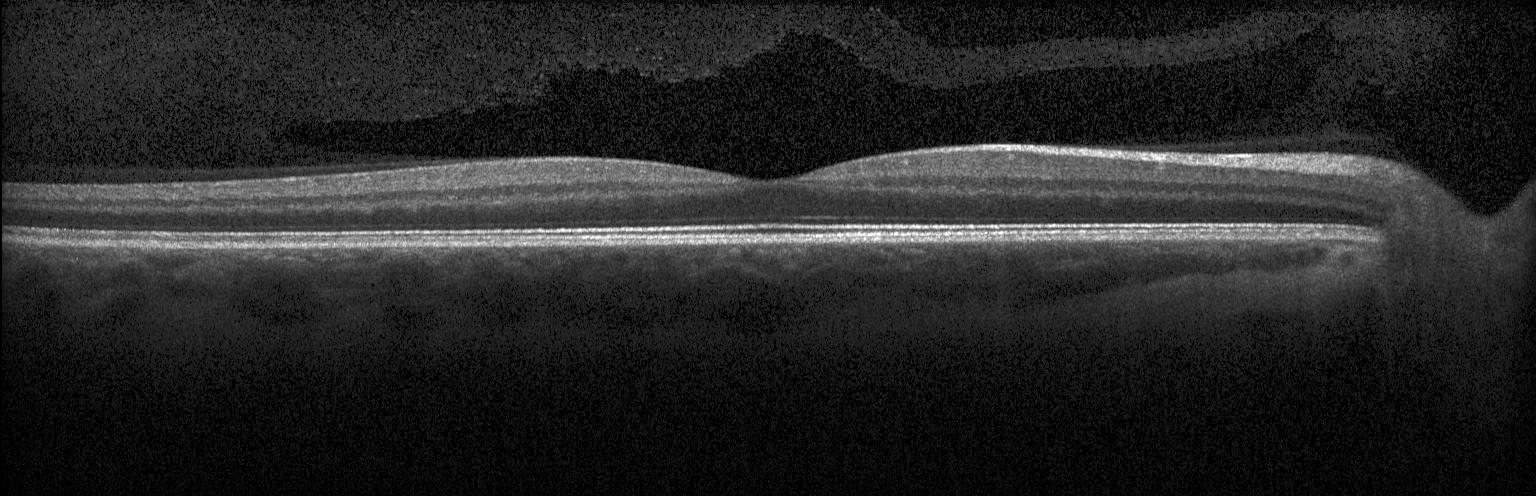 Centered on the fovea. OCT line scan. Spectral-domain OCT. Acquired on a Heidelberg Spectralis.
Finding: neither choroidal neovascularization, diabetic macular edema, nor drusen.